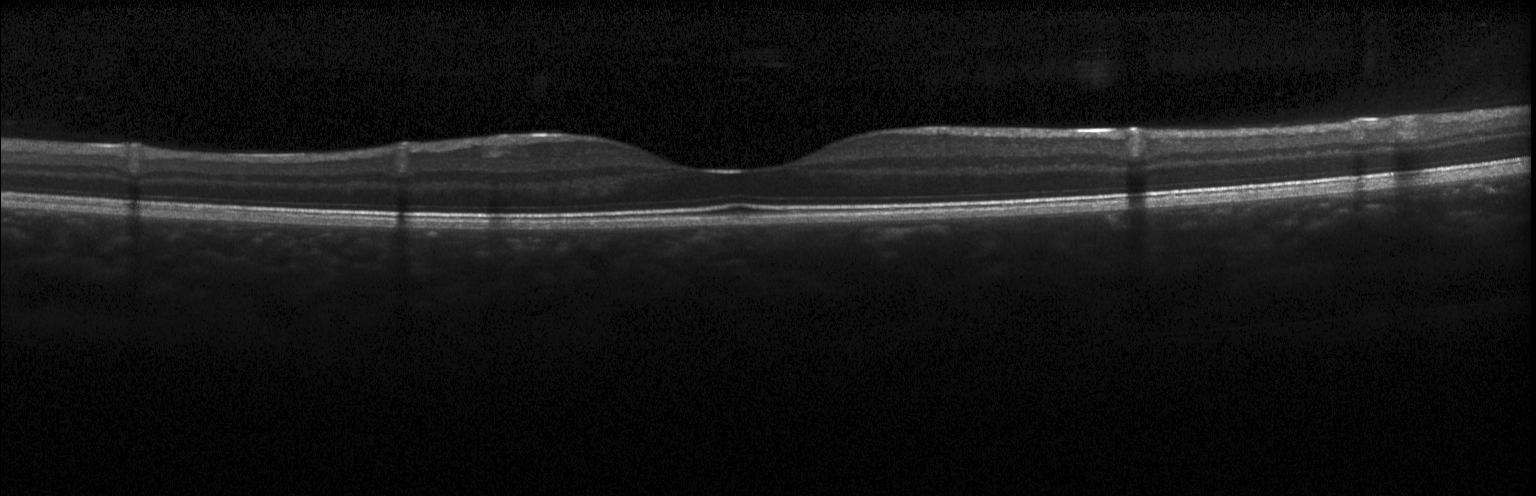
Spectral-domain optical coherence tomography · instrument: Heidelberg Spectralis · retinal OCT B-scan. OCT finding: no choroidal neovascularization, no diabetic macular edema, and no drusen.